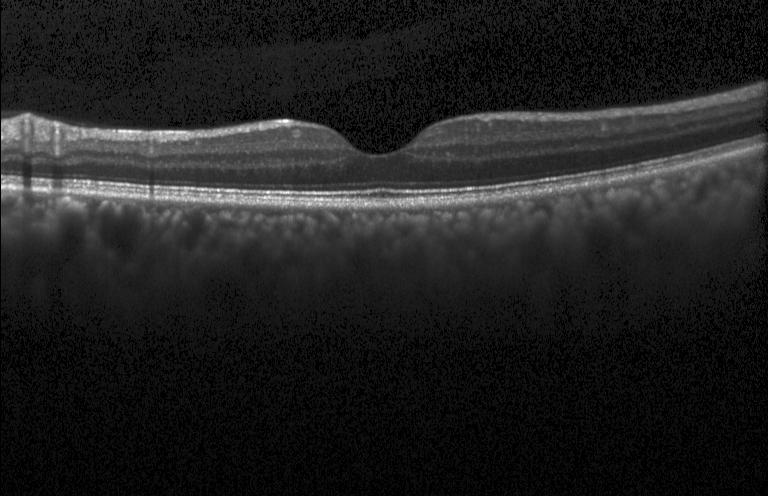
OCT scan showing neither choroidal neovascularization, diabetic macular edema, nor drusen.